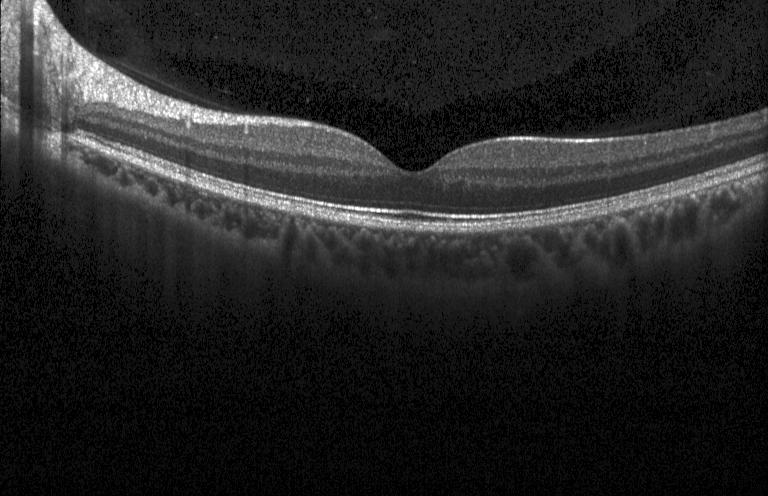
Impression: no choroidal neovascularization, no diabetic macular edema, and no drusen.